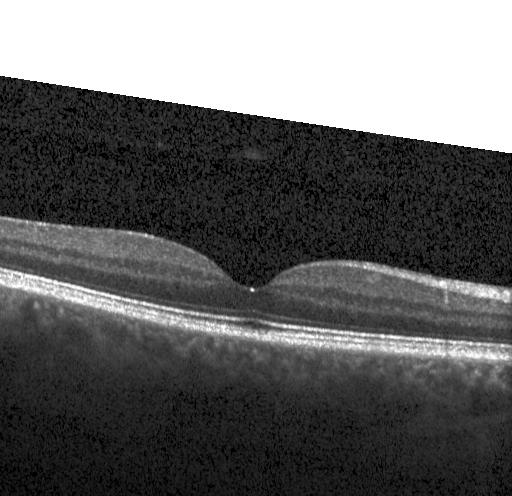
Spectral-domain optical coherence tomography. OCT B-scan
No evidence of choroidal neovascularization, diabetic macular edema, or drusen.